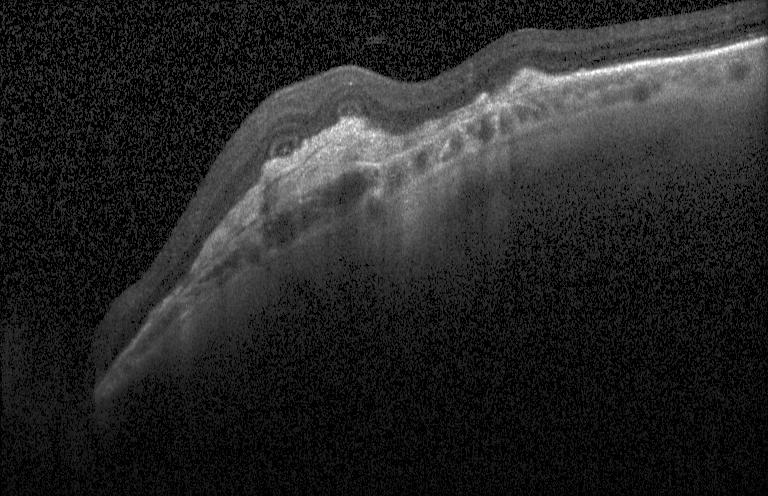

Impression: a choroidal neovascular membrane.